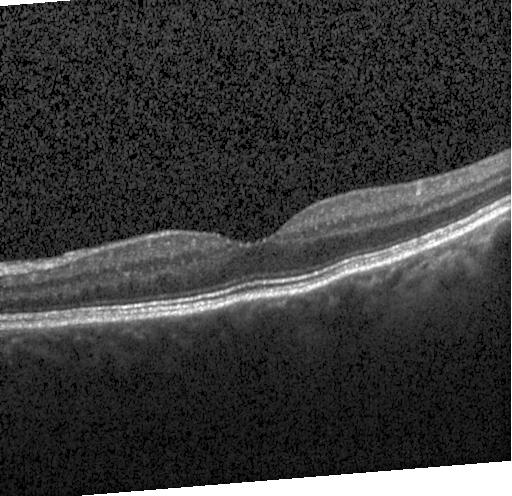
Impression: no CNV, no DME, and no drusen.